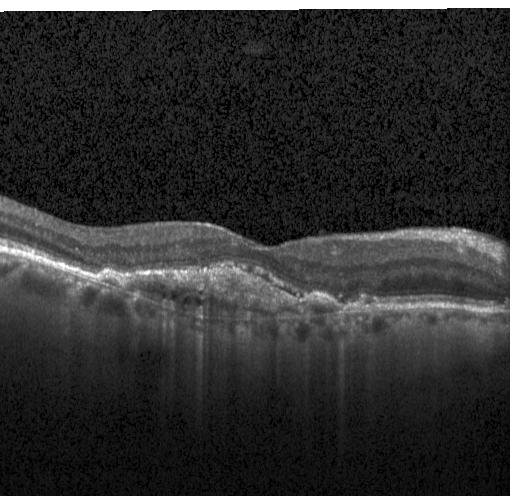
Optical coherence tomography scan, fovea-centered. CNV.